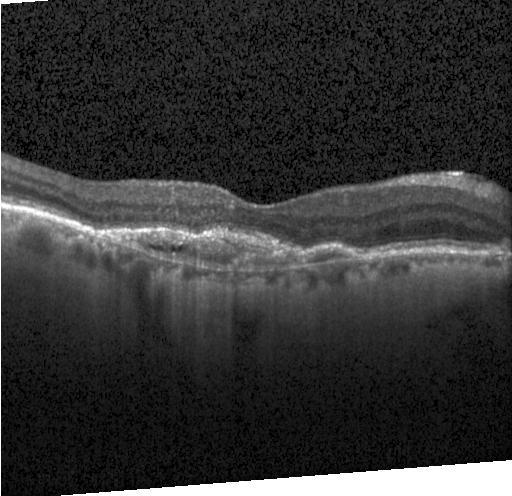
Optical coherence tomography scan. Centered on the fovea.
Assessment: choroidal neovascularization (CNV).